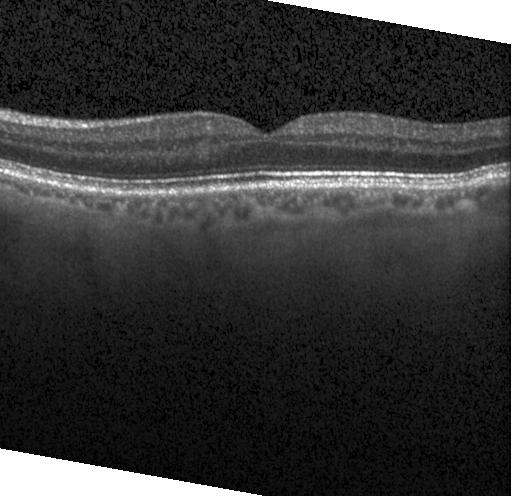
Through the macula; SD-OCT; optical coherence tomography scan
This B-scan demonstrates no choroidal neovascularization, no diabetic macular edema, and no drusen.